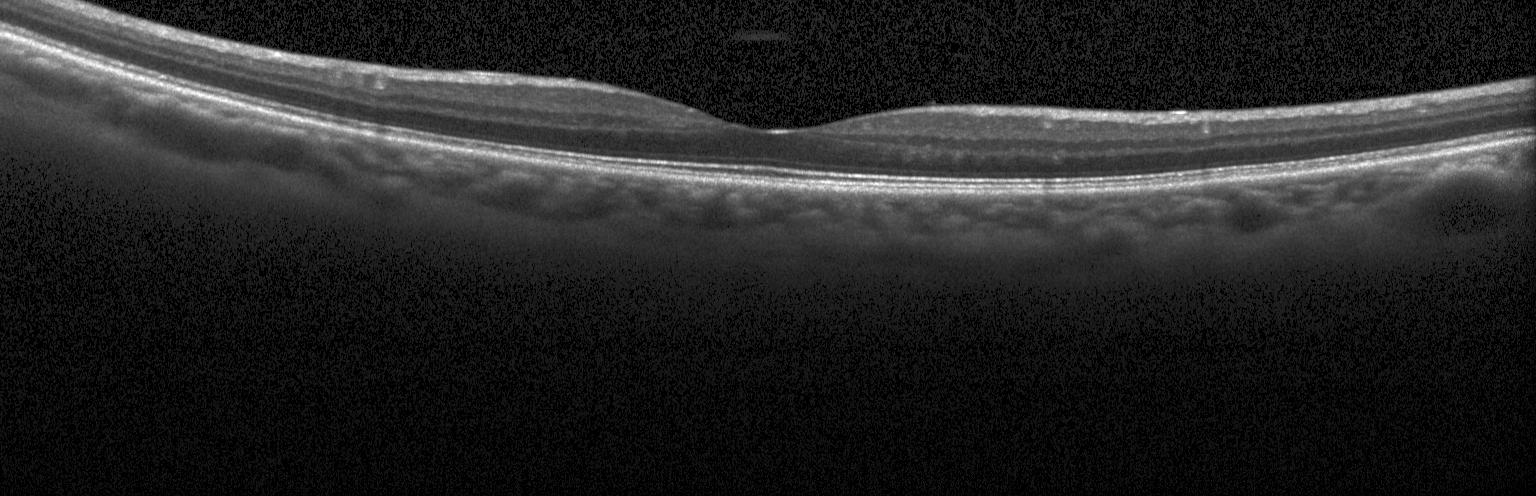
Optical coherence tomography scan. Macular scan. Instrument: Heidelberg Spectralis. SD-OCT
The scan shows no choroidal neovascularization, no diabetic macular edema, and no drusen.